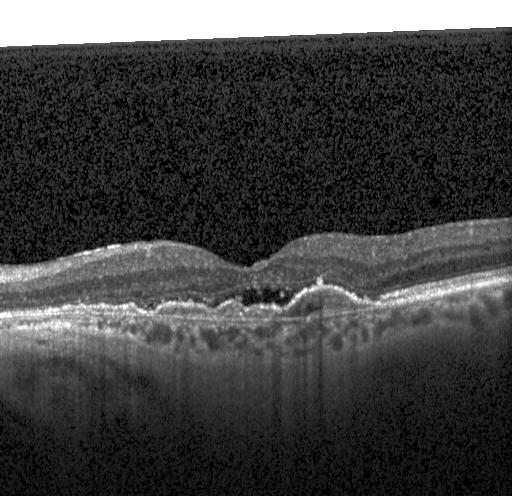

Optical coherence tomography scan — Choroidal neovascularization.